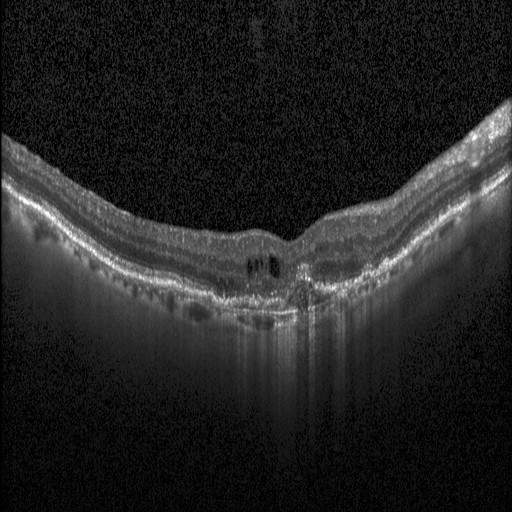 Retinal OCT cross-section.
Diabetic macular edema (DME).